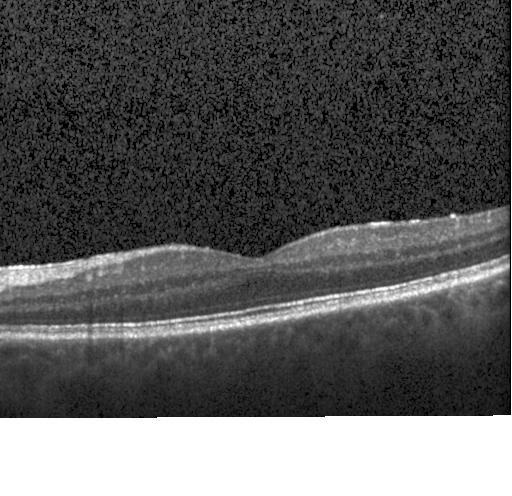

Spectral-domain OCT. Instrument: Heidelberg Spectralis. Optical coherence tomography B-scan — Diagnosis: no choroidal neovascularization, diabetic macular edema, or drusen.